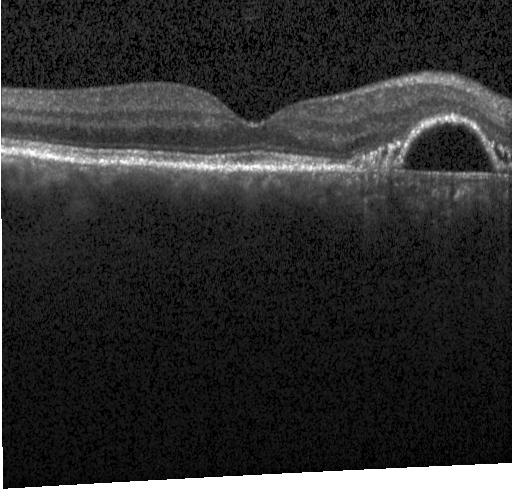

Horizontal scan through the fovea; instrument: Heidelberg Spectralis; retinal OCT cross-section; SD-OCT.
Assessment: choroidal neovascularization.